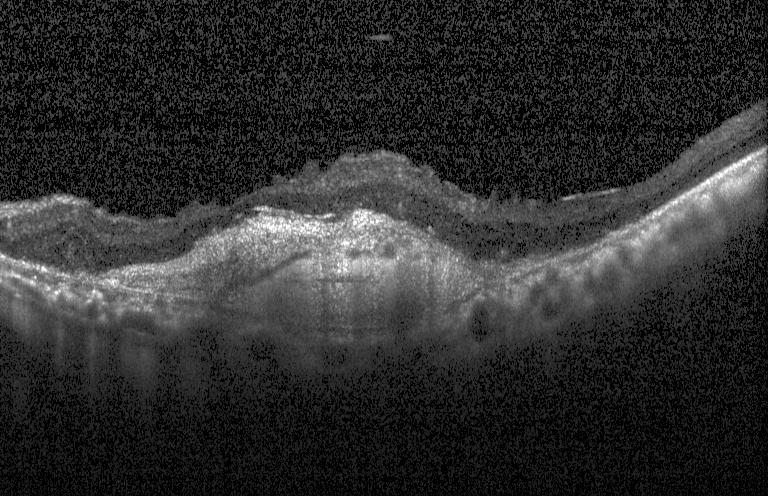

Finding: CNV.